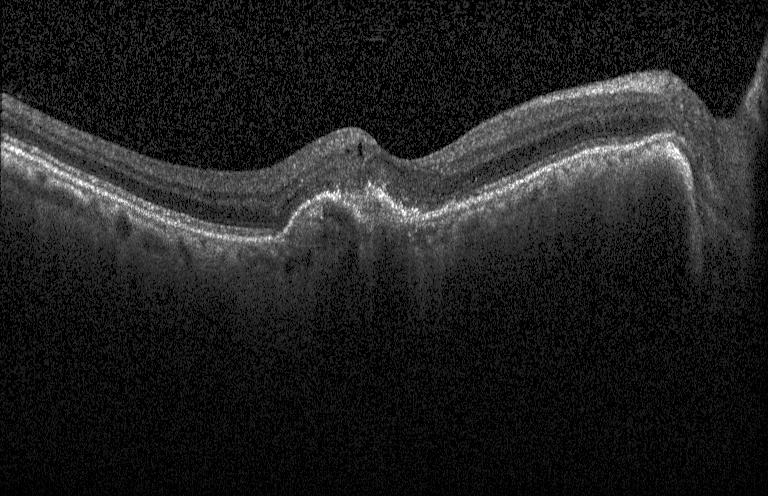
Retinal OCT B-scan
Diagnosis: a choroidal neovascular membrane.